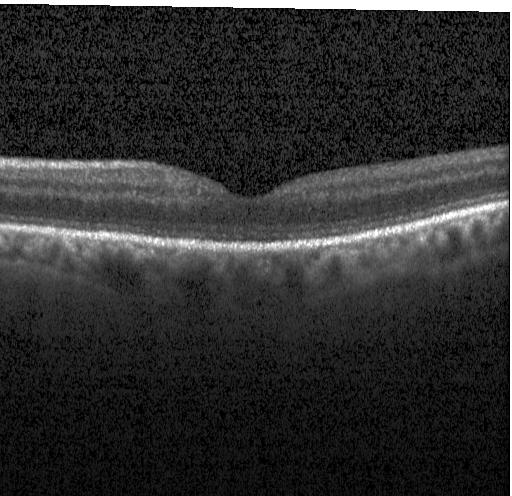

Acquired on a Heidelberg Spectralis. Optical coherence tomography B-scan
The scan shows no choroidal neovascularization, diabetic macular edema, or drusen.